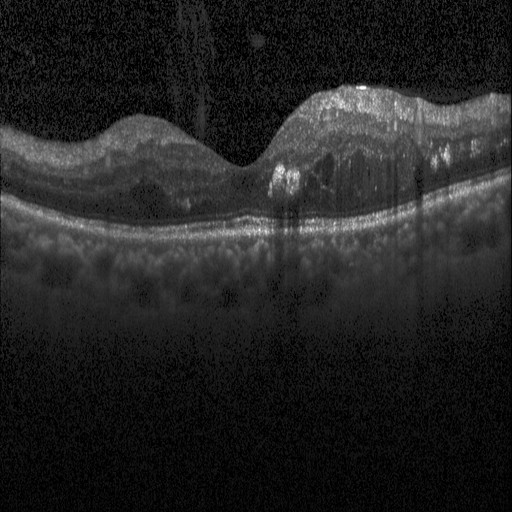
Spectral-domain OCT · optical coherence tomography scan — Assessment: diabetic macular edema (DME).